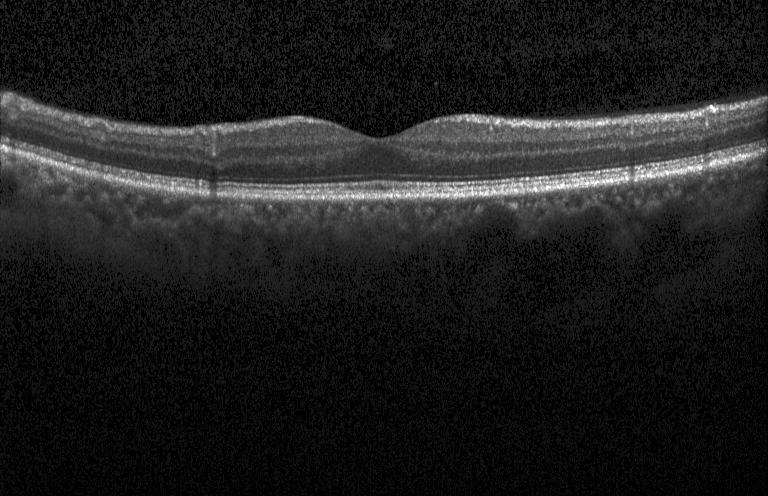 Macular scan; optical coherence tomography B-scan — OCT finding: neither choroidal neovascularization, diabetic macular edema, nor drusen.